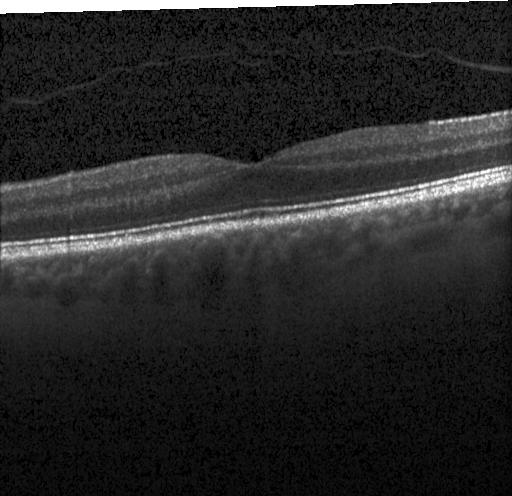
Impression: no choroidal neovascularization, no diabetic macular edema, and no drusen.